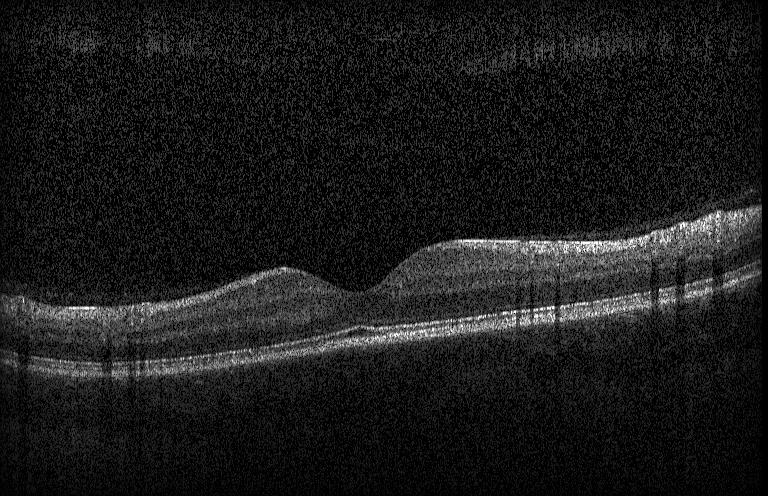

Dx: neither CNV, DME, nor drusen.